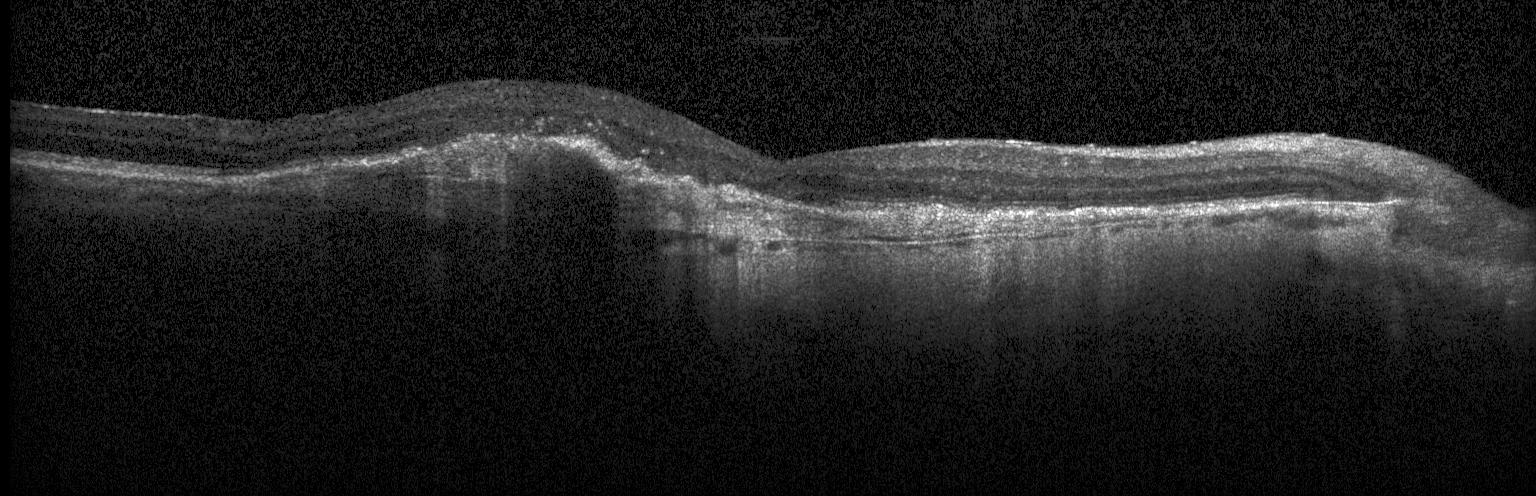

Optical coherence tomography scan · spectral-domain optical coherence tomography · fovea-centered · instrument: Heidelberg Spectralis. Assessment: a choroidal neovascular membrane.